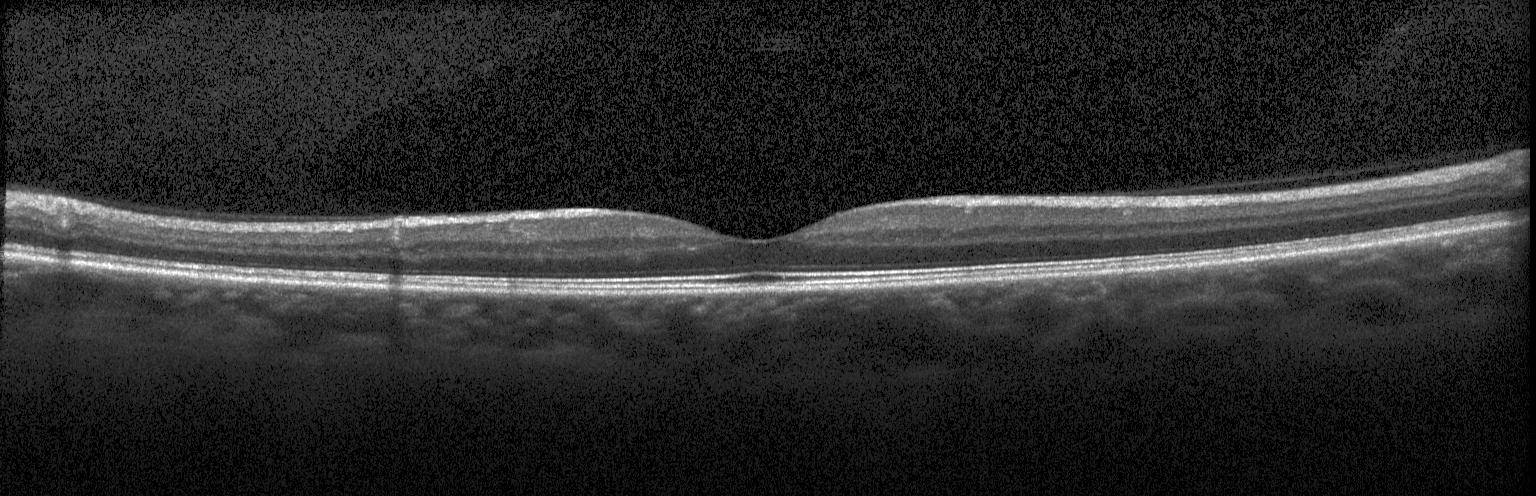
Retinal OCT cross-section; spectral-domain optical coherence tomography
OCT finding: no CNV, DME, or drusen.